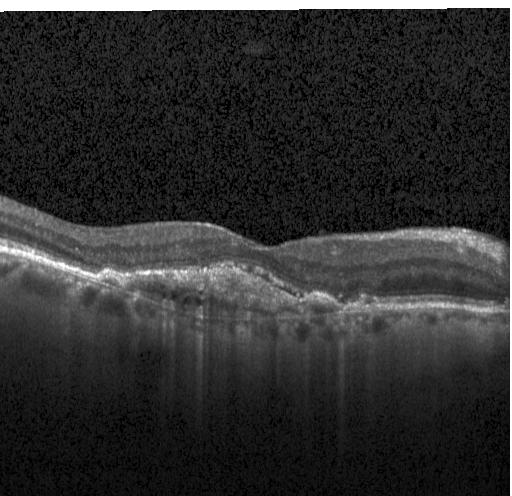 Horizontal scan through the fovea, retinal OCT cross-section, spectral-domain optical coherence tomography, instrument: Heidelberg Spectralis. Macular OCT: a choroidal neovascular membrane.